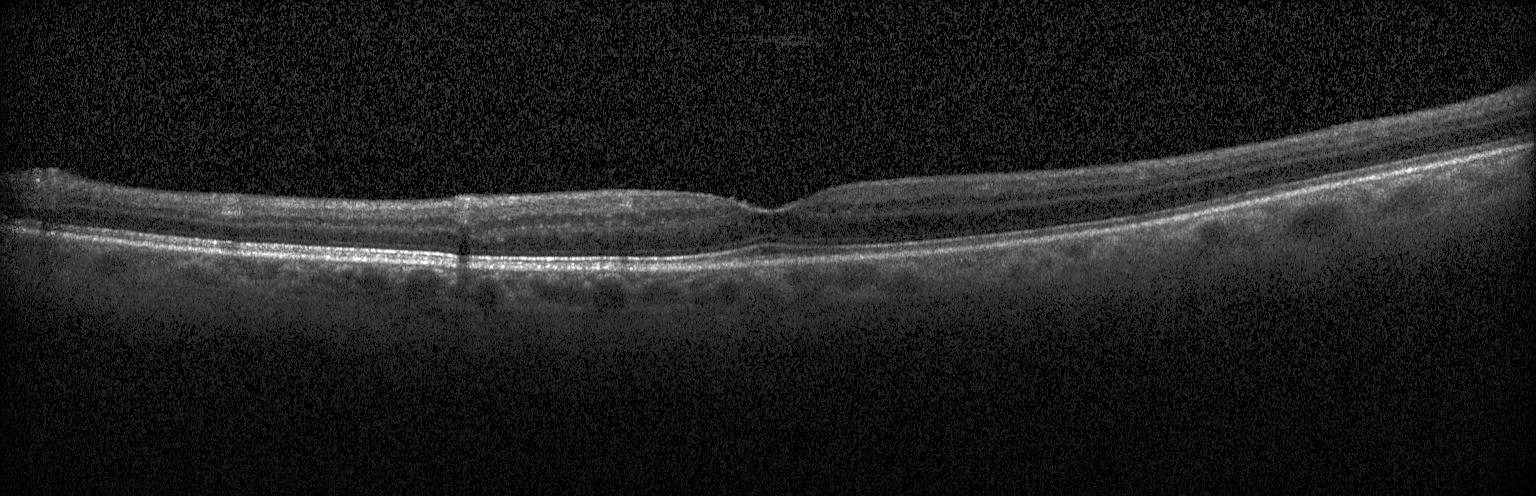 Neither CNV, DME, nor drusen.